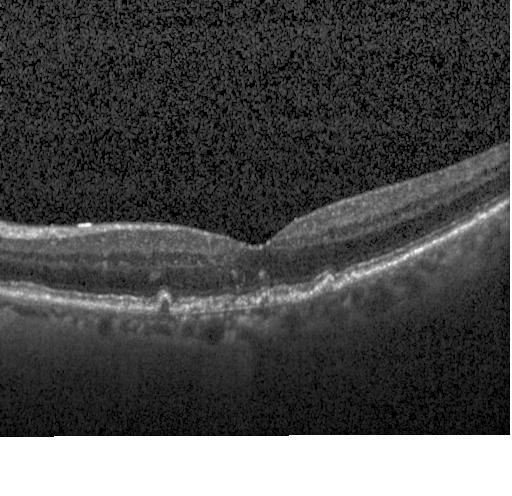

Impression: sub-RPE drusenoid deposits.